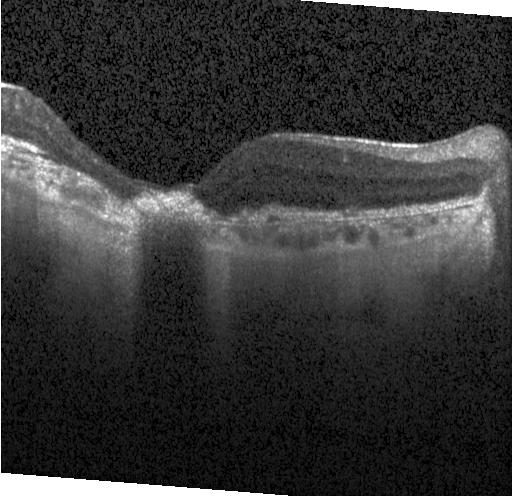
Diagnosis: choroidal neovascularization (CNV).